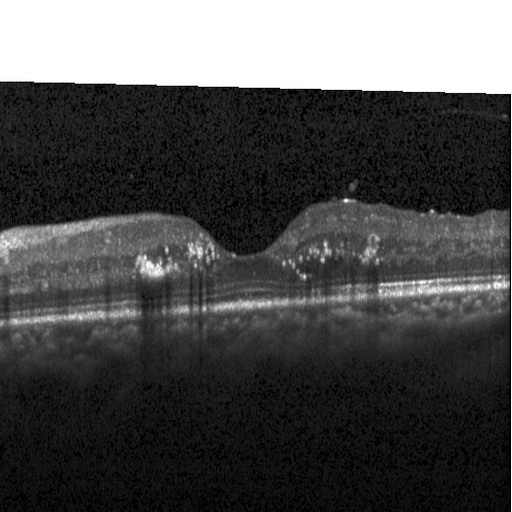
Retinal OCT cross-section showing DME.